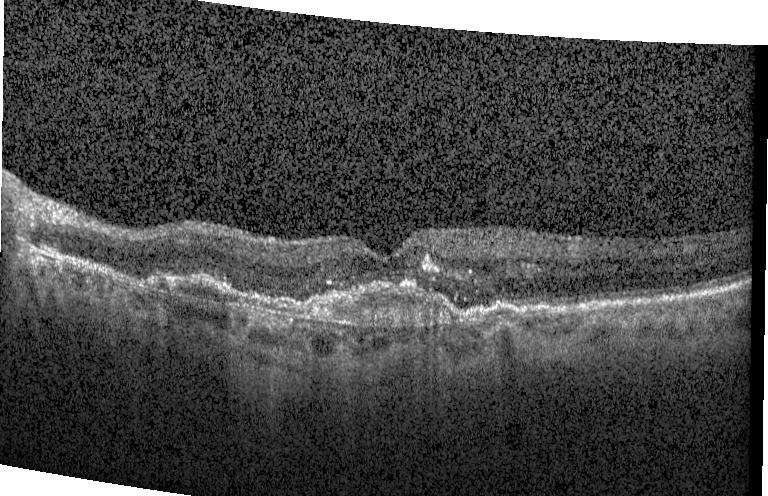

Instrument: Heidelberg Spectralis. Spectral-domain OCT. Retinal OCT cross-section — Diagnosis: choroidal neovascularization (CNV).